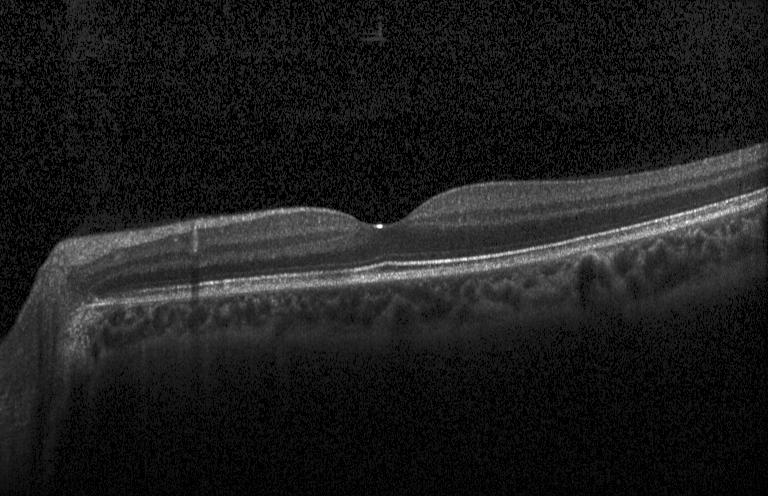
Retinal OCT cross-section — Diagnosis: no evidence of CNV, DME, or drusen.